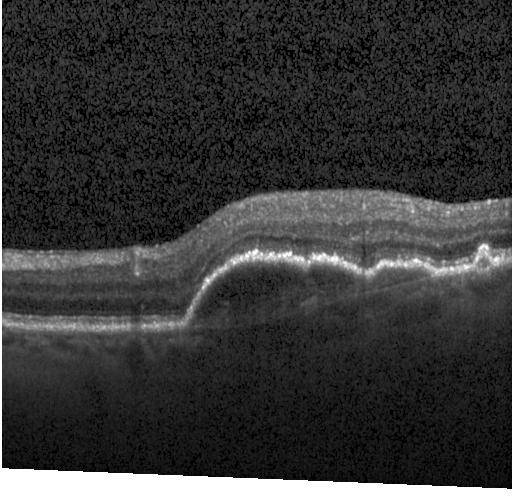 Fovea-centered. Spectral-domain OCT. Heidelberg Spectralis. OCT B-scan.
A choroidal neovascular membrane.